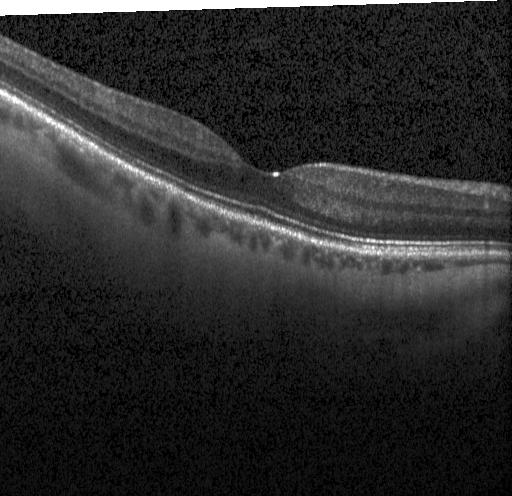 Heidelberg Spectralis; SD-OCT; optical coherence tomography scan; through the macula
This B-scan demonstrates no choroidal neovascularization, diabetic macular edema, or drusen.